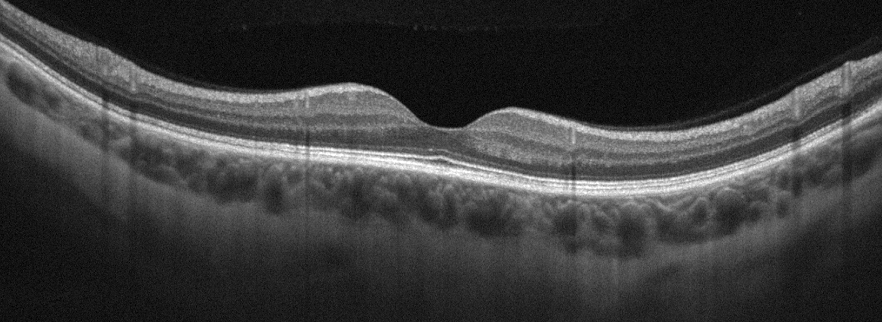
OCT line scan, OS. Finding: no AMD, DME, ERM, RAO, RVO, or VID.